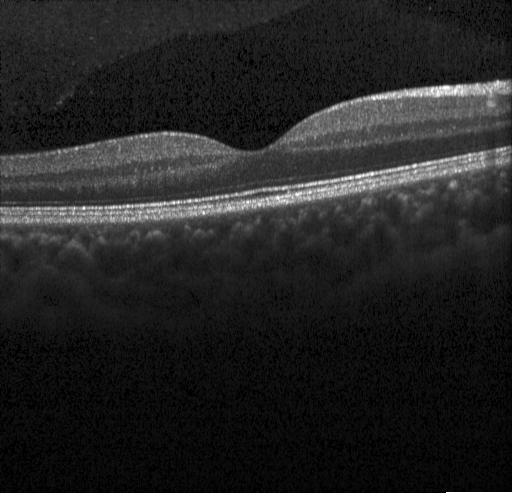 Fovea-centered · retinal OCT cross-section · SD-OCT · acquired on a Heidelberg Spectralis — Impression: no choroidal neovascularization, no diabetic macular edema, and no drusen.